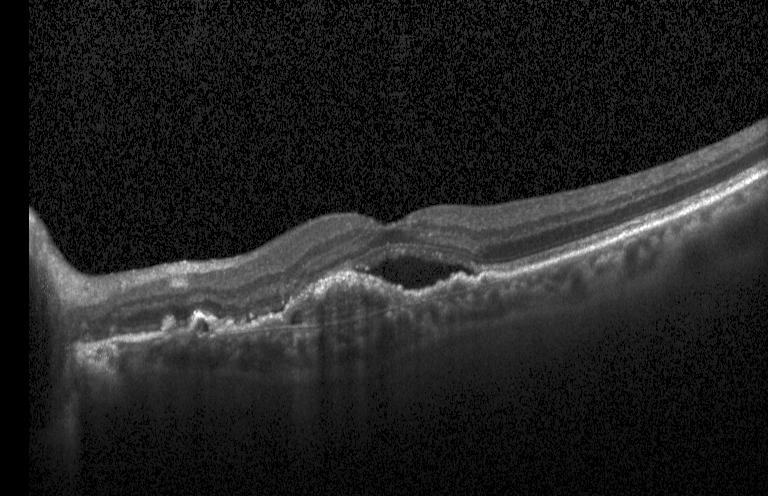
Spectral-domain OCT · retinal OCT B-scan · fovea-centered · acquired on a Heidelberg Spectralis — Macular OCT: a choroidal neovascular membrane.